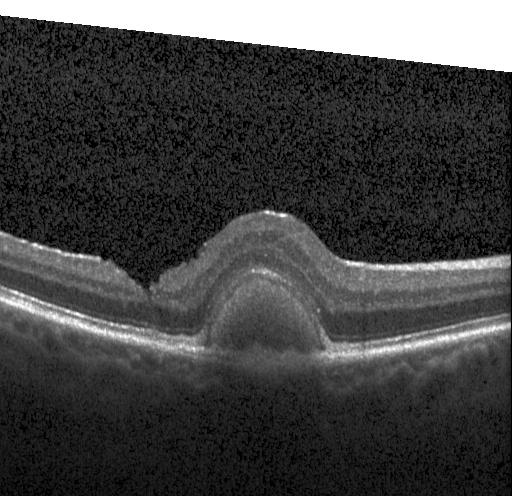
SD-OCT, OCT line scan, horizontal scan through the fovea. OCT finding: choroidal neovascularization (CNV).